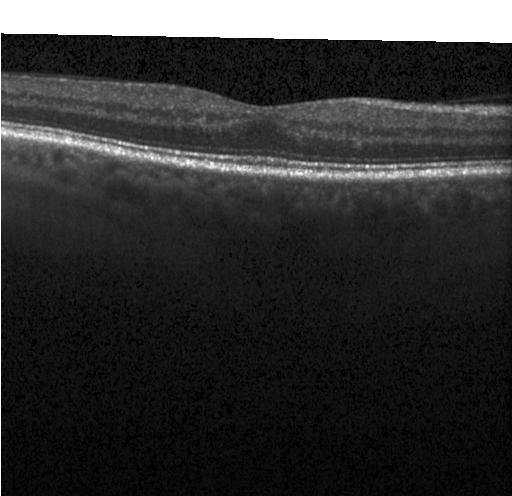
Impression: no evidence of choroidal neovascularization, diabetic macular edema, or drusen.